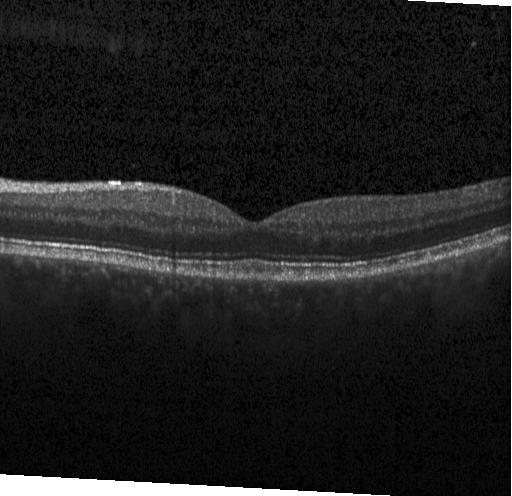

Heidelberg Spectralis · spectral-domain OCT · OCT line scan.
This B-scan demonstrates no choroidal neovascularization, diabetic macular edema, or drusen.